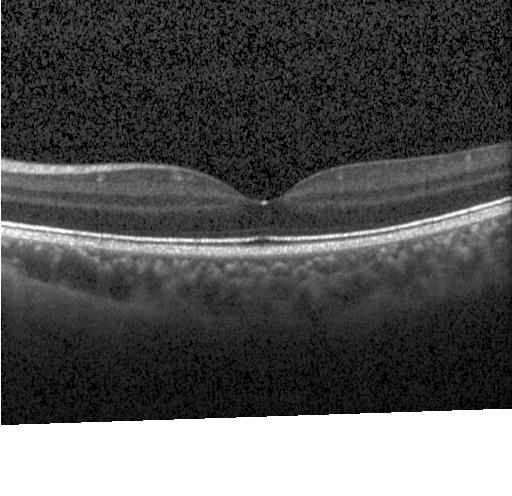
Diagnosis: no evidence of choroidal neovascularization, diabetic macular edema, or drusen.